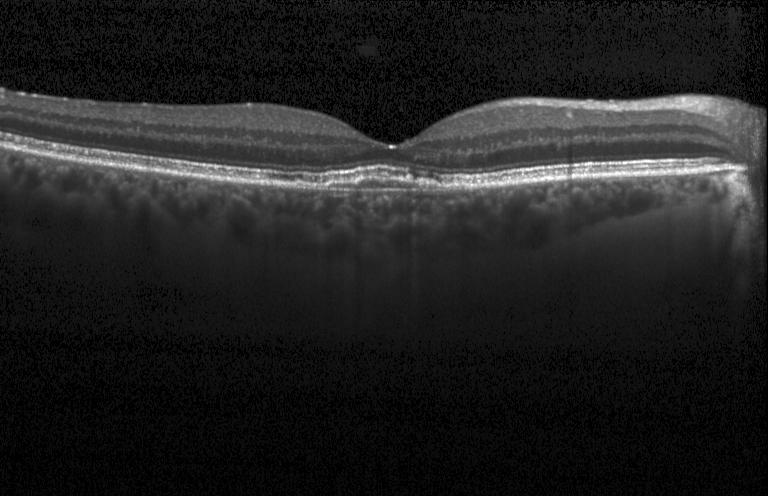

OCT B-scan — Dx: CNV.